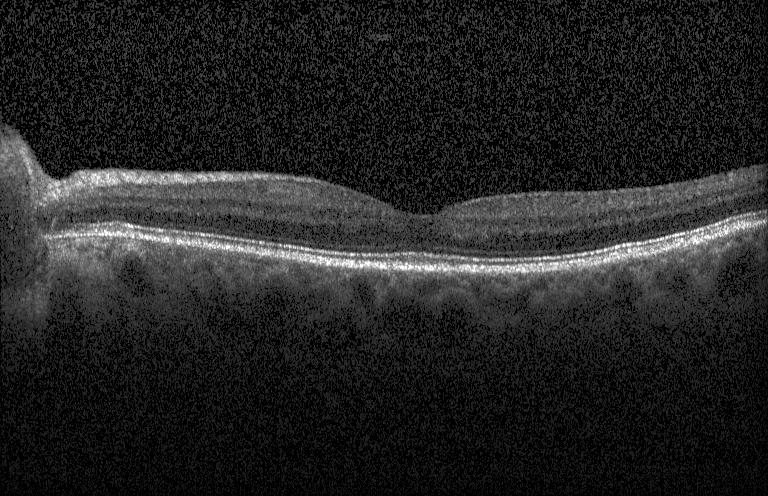 Optical coherence tomography B-scan — Macular OCT: no CNV, DME, or drusen.